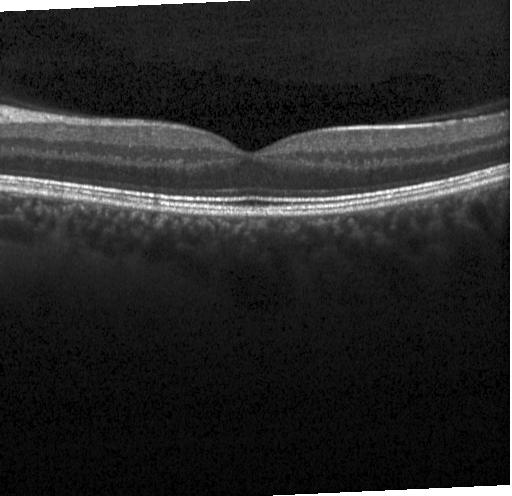 OCT B-scan, macular scan, spectral-domain OCT, acquired on a Heidelberg Spectralis
Impression: no choroidal neovascularization, diabetic macular edema, or drusen.